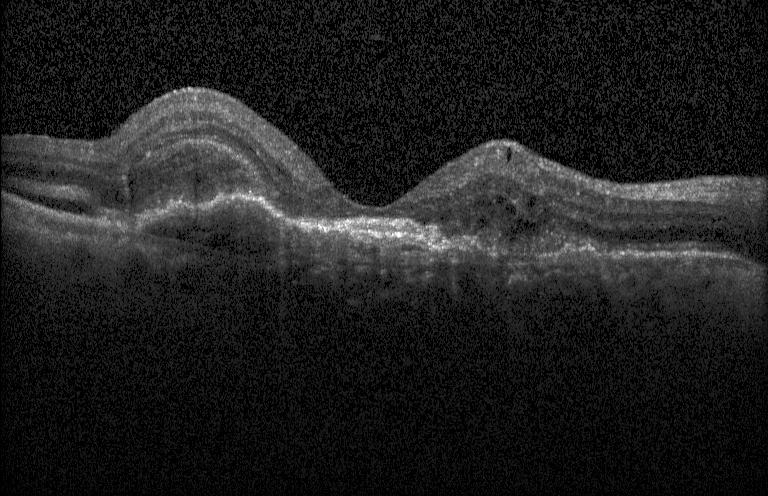
Optical coherence tomography scan; Heidelberg Spectralis; spectral-domain optical coherence tomography; fovea-centered
Diagnosis: a choroidal neovascular membrane.